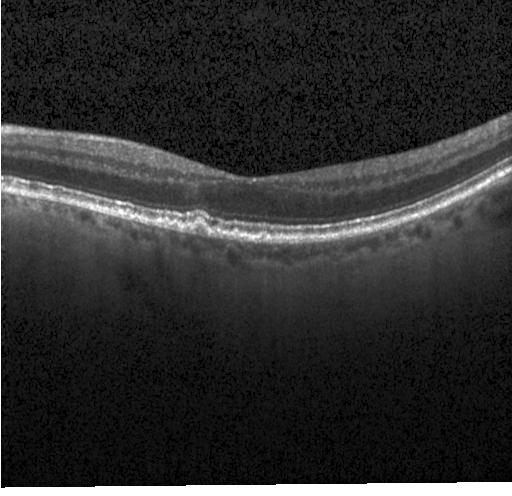

Instrument: Heidelberg Spectralis; through the macula; optical coherence tomography scan; spectral-domain optical coherence tomography.
Dx: multiple drusen.